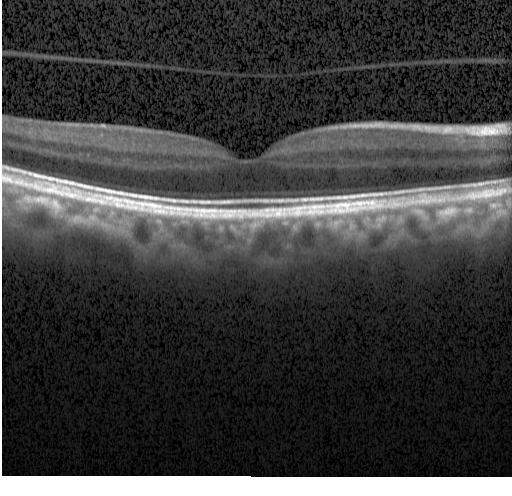

Macular OCT demonstrating no evidence of choroidal neovascularization, diabetic macular edema, or drusen.